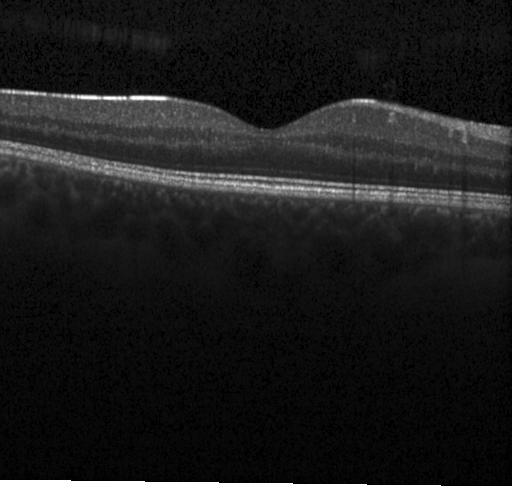 SD-OCT, retinal OCT cross-section.
OCT finding: no choroidal neovascularization, no diabetic macular edema, and no drusen.